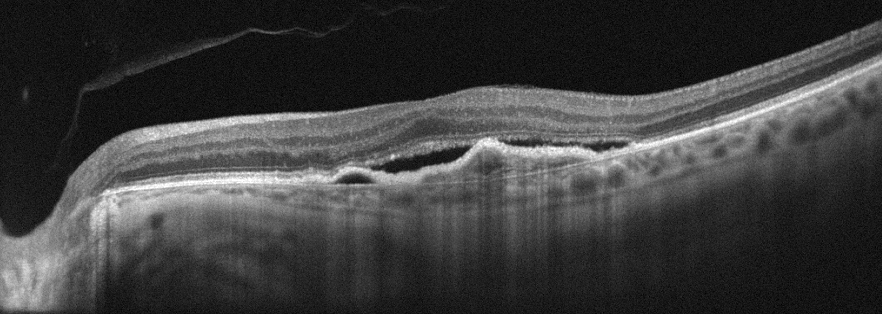 Retinal OCT B-scan · left eye.
Finding: AMD.